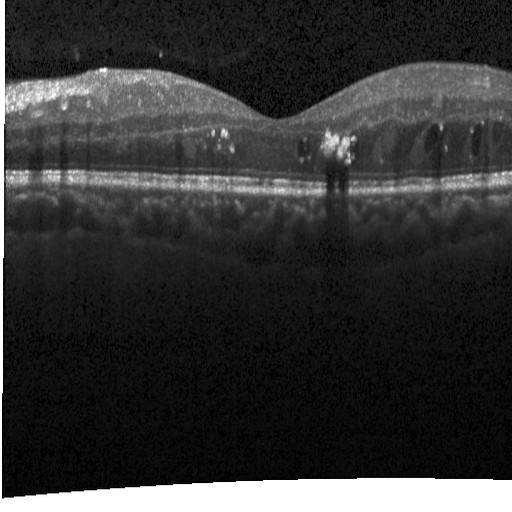 Retinal OCT cross-section showing diabetic macular edema (DME).